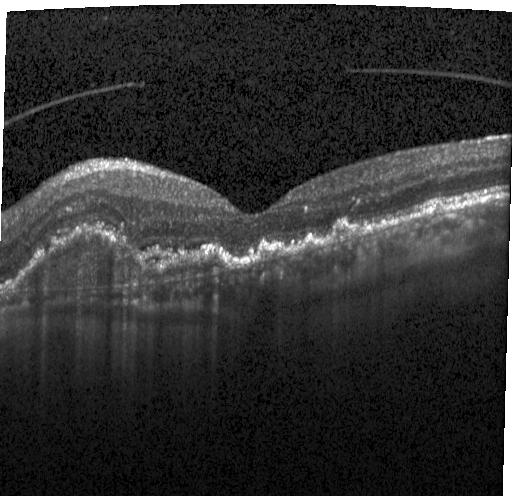

OCT line scan; fovea-centered — Impression: a choroidal neovascular membrane.